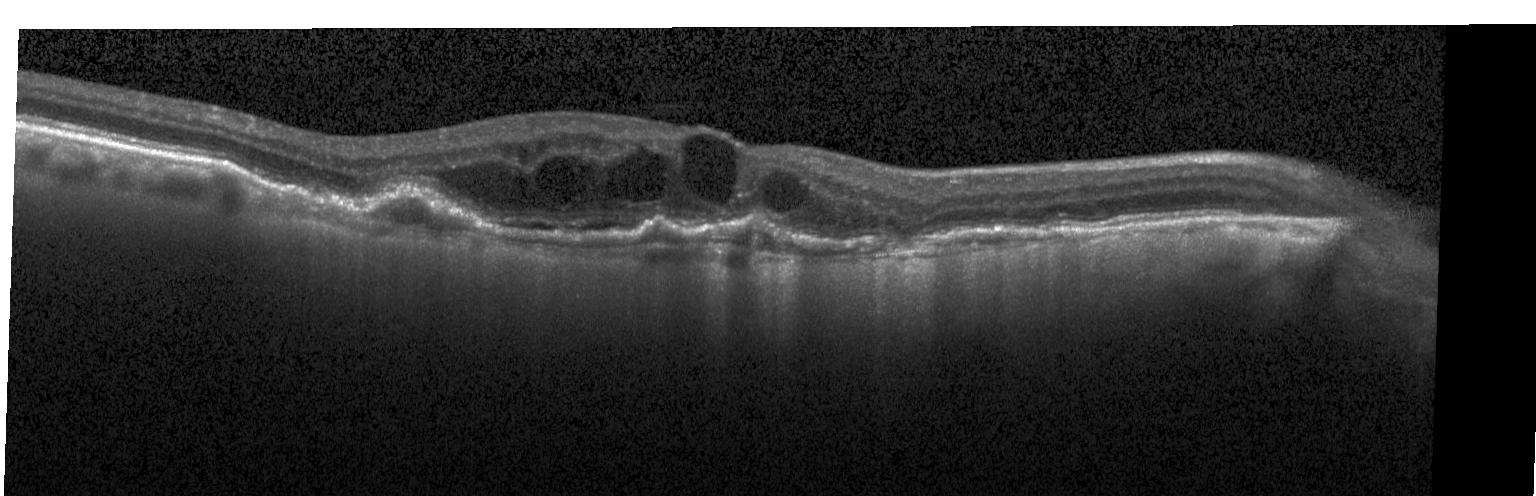 Fovea-centered · acquired on a Heidelberg Spectralis · optical coherence tomography scan · spectral-domain optical coherence tomography. Dx: a choroidal neovascular membrane.